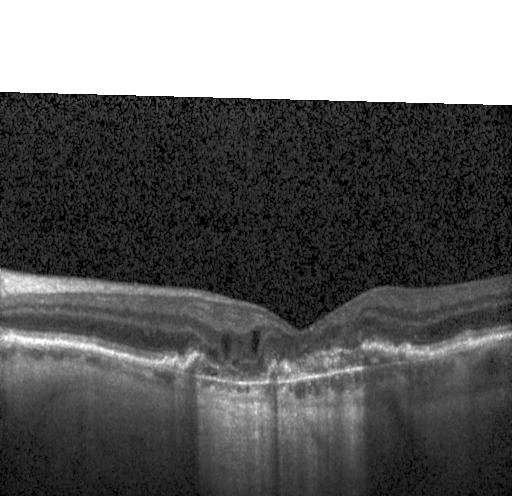

Finding: a choroidal neovascular membrane.